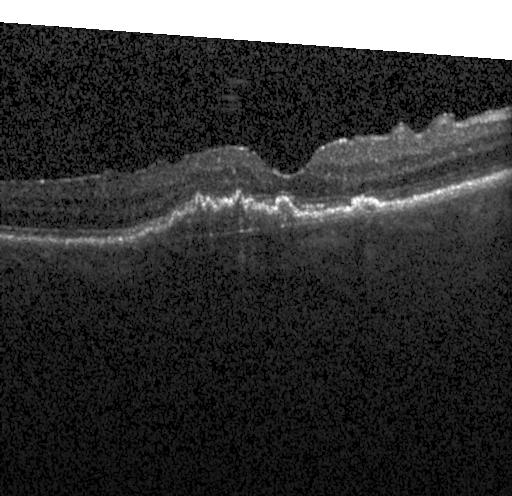
Retinal OCT cross-section showing a choroidal neovascular membrane.